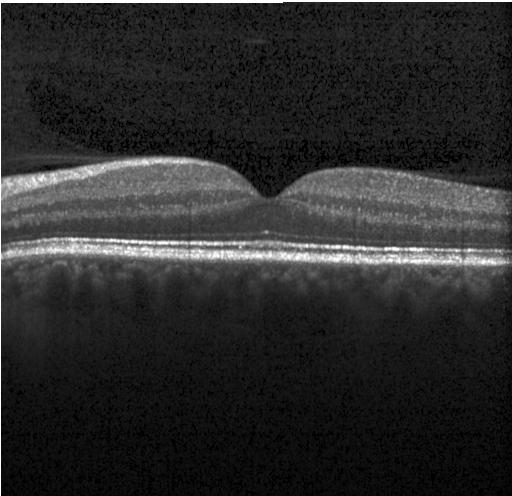
Optical coherence tomography scan.
Assessment: neither choroidal neovascularization, diabetic macular edema, nor drusen.